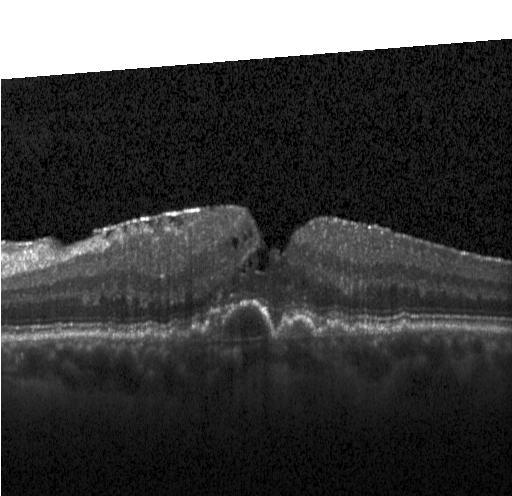 Retinal OCT B-scan — This B-scan demonstrates CNV.